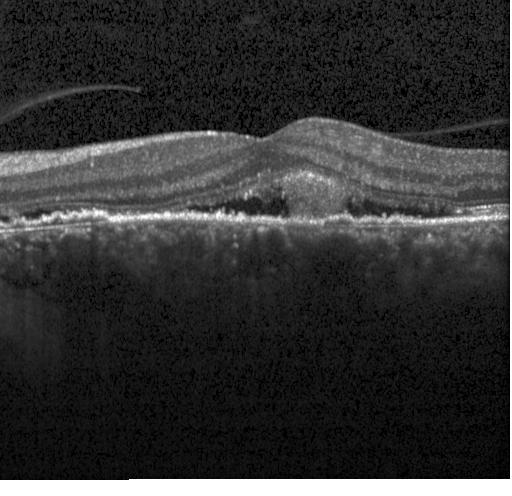

OCT finding: choroidal neovascularization.